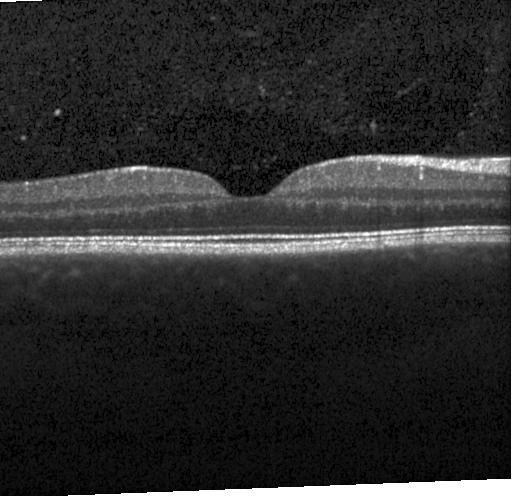

Retinal OCT B-scan
The scan shows no choroidal neovascularization, diabetic macular edema, or drusen.